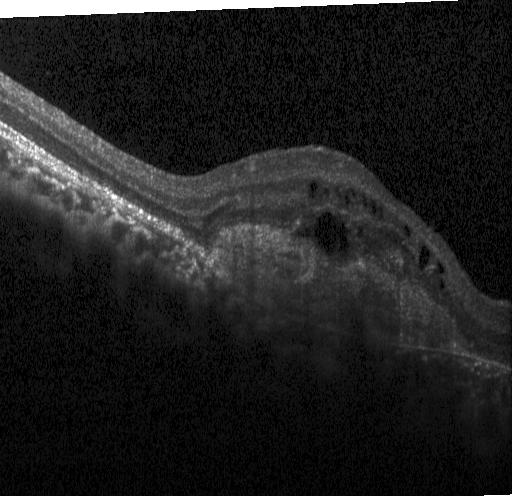 OCT line scan — Macular OCT: a choroidal neovascular membrane.